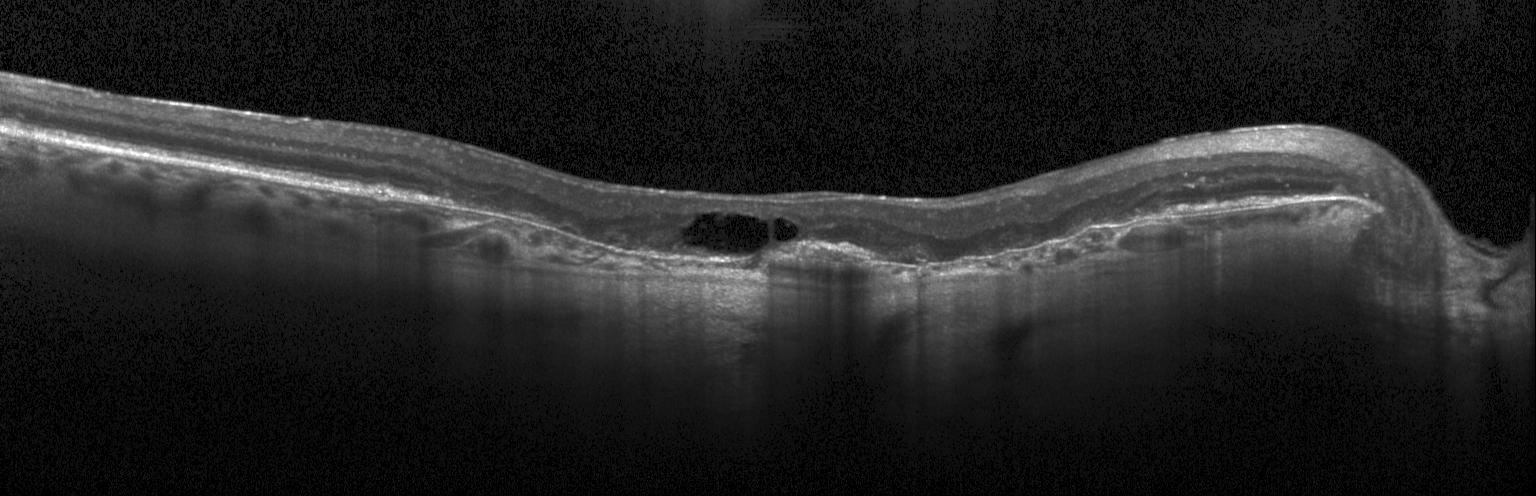 OCT B-scan
Impression: a choroidal neovascular membrane.